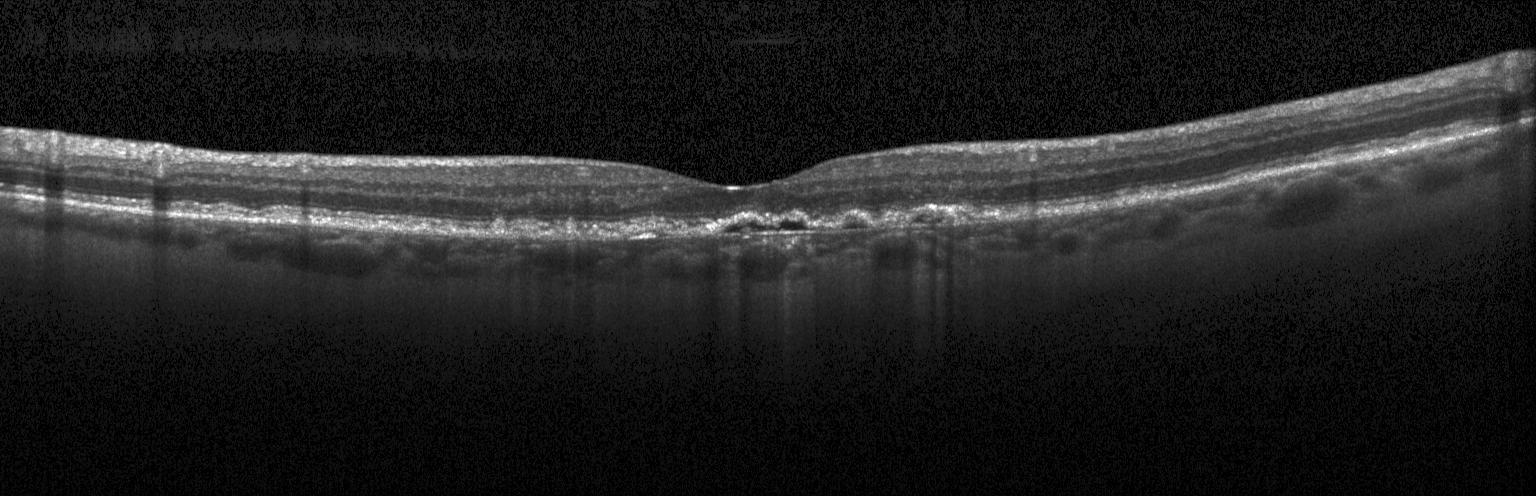 Optical coherence tomography scan. Heidelberg Spectralis. Spectral-domain OCT
Finding: choroidal neovascularization.